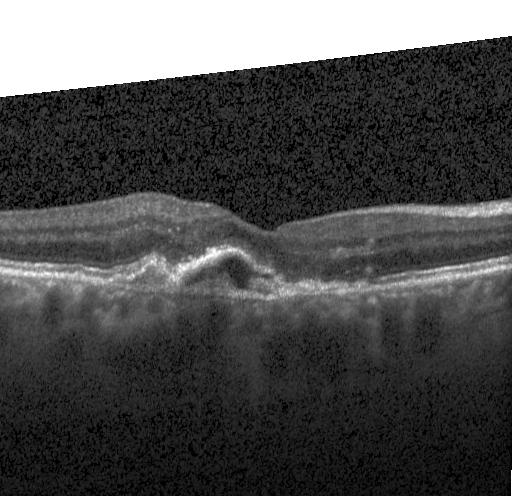

Impression: choroidal neovascularization.